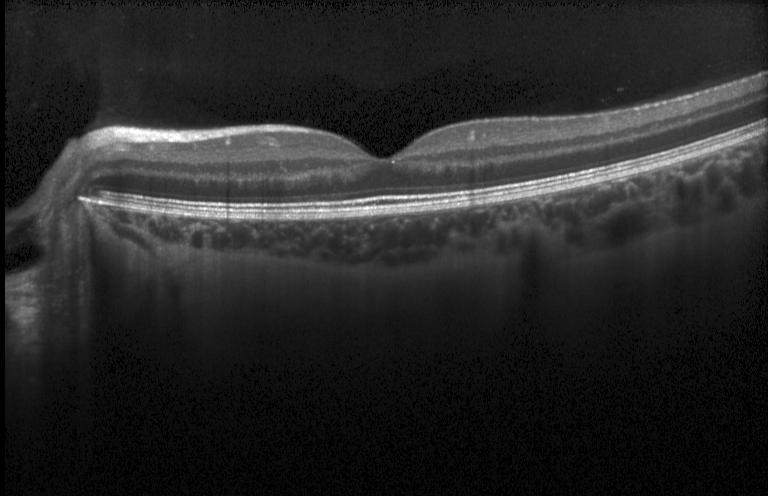

Neither choroidal neovascularization, diabetic macular edema, nor drusen.